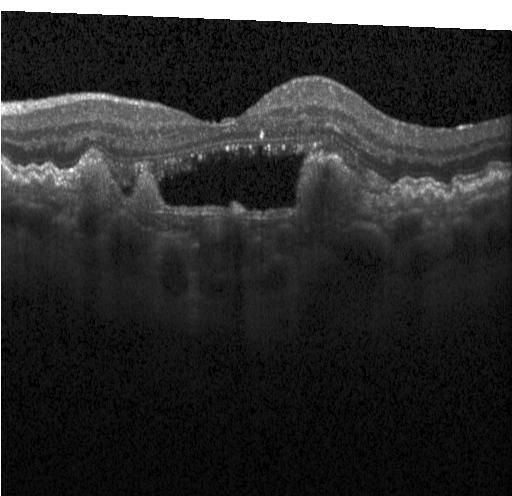
OCT finding: a choroidal neovascular membrane.